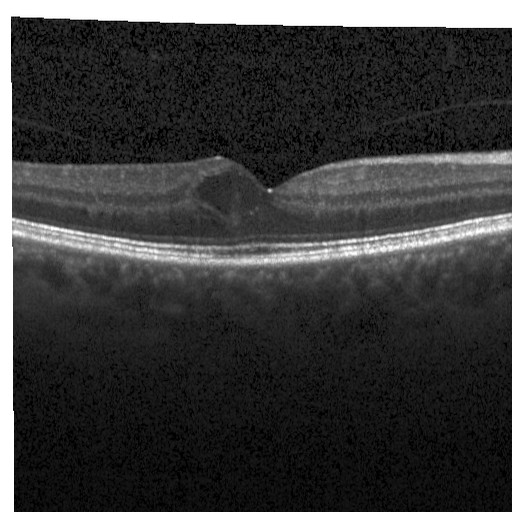

OCT line scan
Diagnosis: diabetic macular edema (DME).